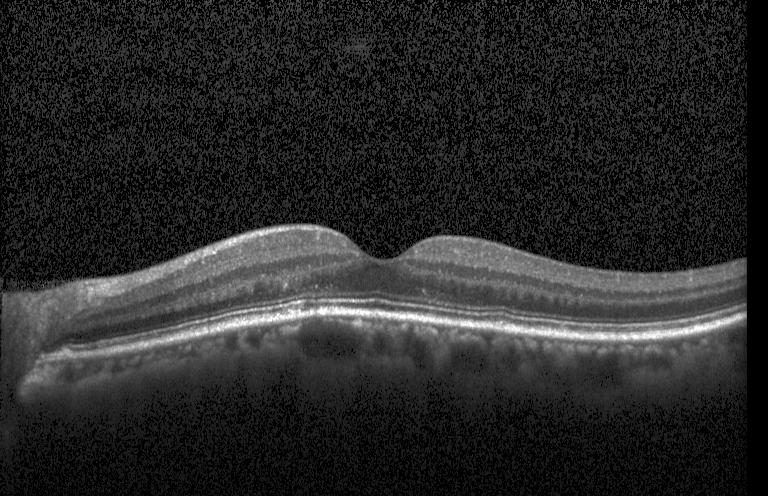
The scan shows no choroidal neovascularization, diabetic macular edema, or drusen.